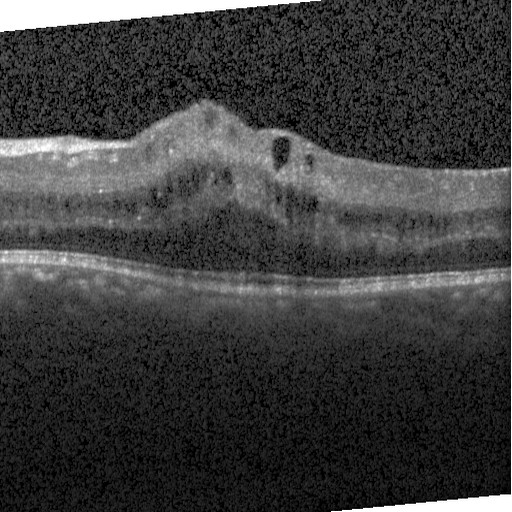
Retinal OCT B-scan; fovea-centered — Impression: diabetic macular edema (DME).